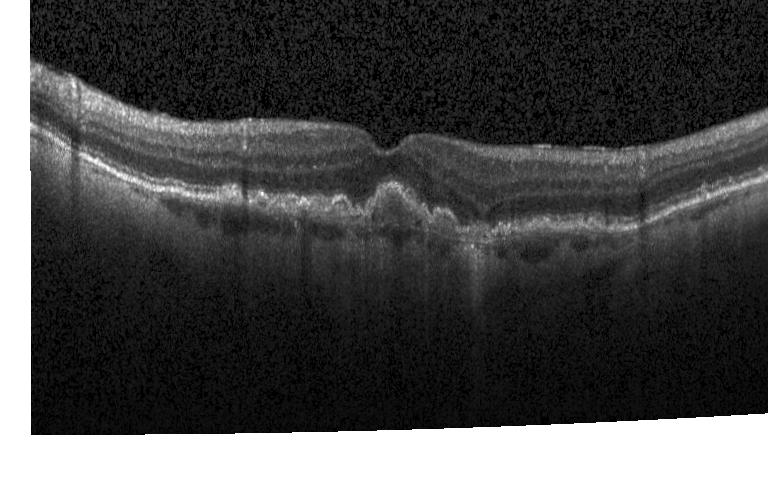
Retinal OCT cross-section · Heidelberg Spectralis OCT system · horizontal scan through the fovea — The scan shows a choroidal neovascular membrane.